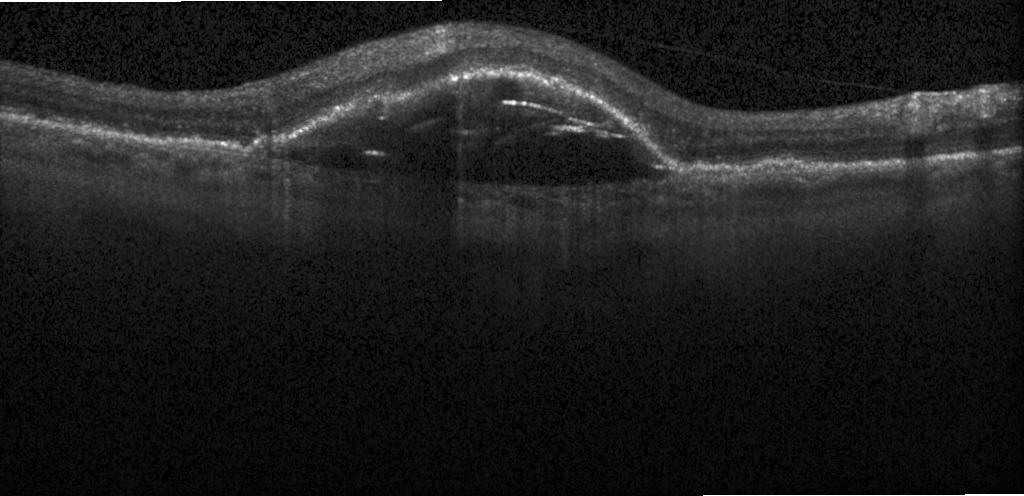

Spectral-domain optical coherence tomography, Heidelberg Spectralis, optical coherence tomography B-scan, centered on the fovea. Impression: choroidal neovascularization (CNV).